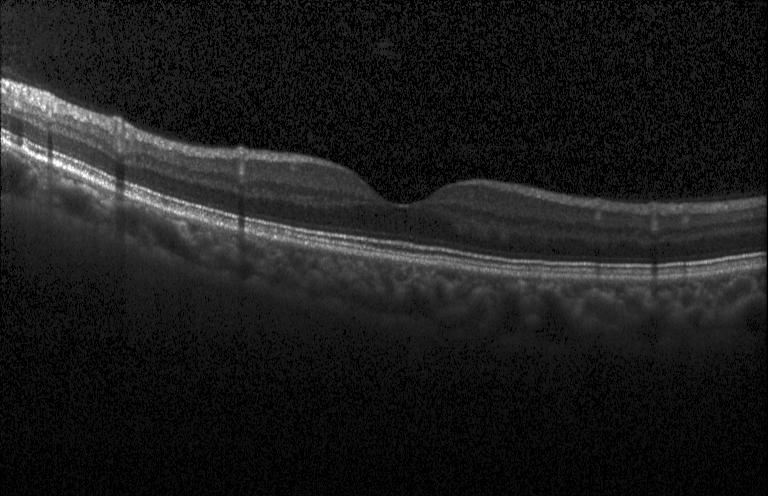

Macular OCT: neither choroidal neovascularization, diabetic macular edema, nor drusen.